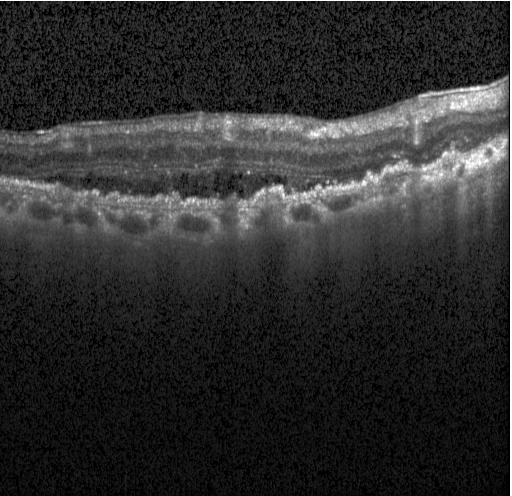

Retinal OCT cross-section.
Assessment: choroidal neovascularization (CNV).